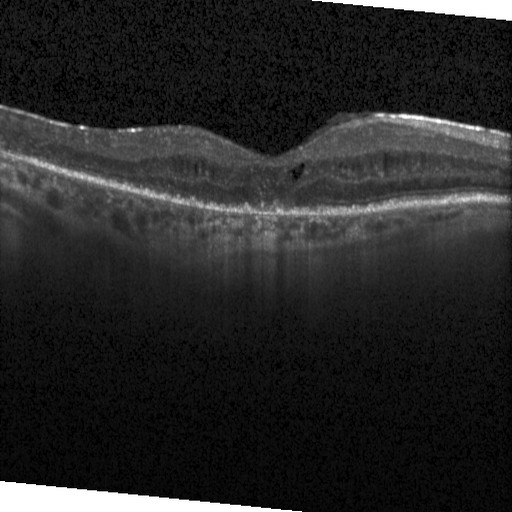 Heidelberg Spectralis. Optical coherence tomography B-scan — The scan shows DME.